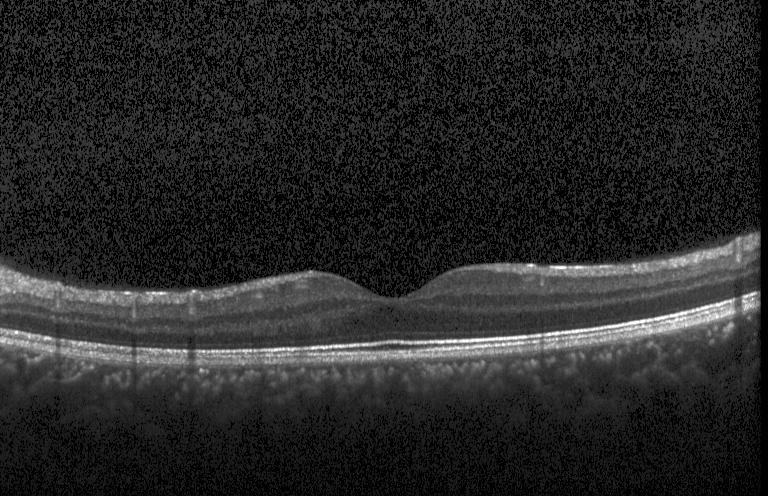
Retinal OCT B-scan. Assessment: neither choroidal neovascularization, diabetic macular edema, nor drusen.